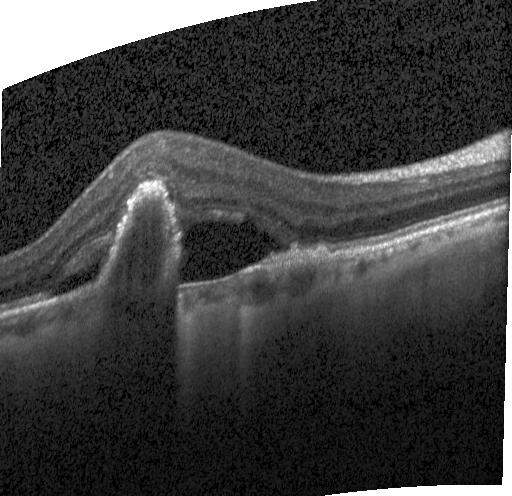 Retinal OCT cross-section. SD-OCT — This B-scan demonstrates choroidal neovascularization.